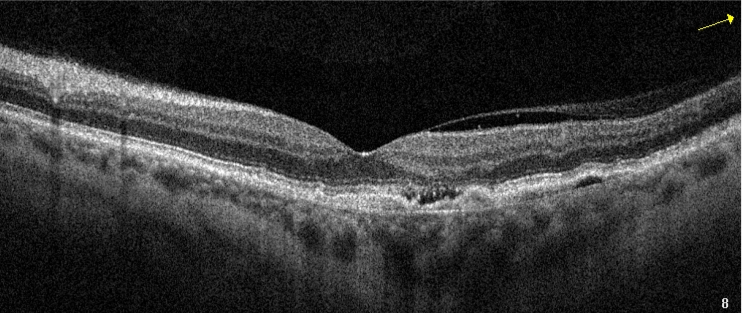
OCT finding: AMD.